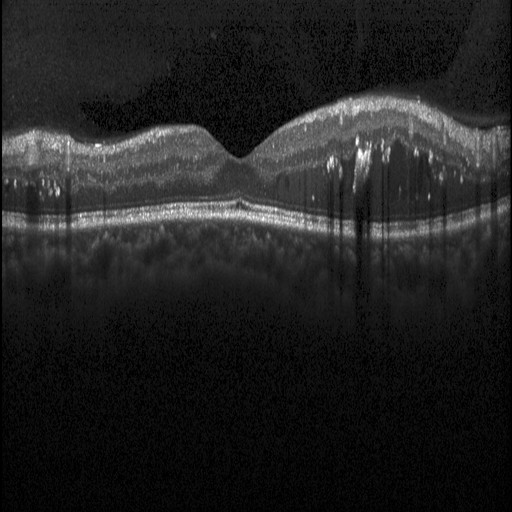 Impression: DME.